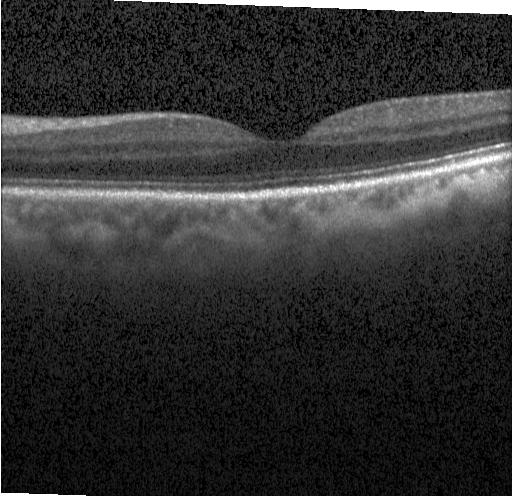
Spectral-domain optical coherence tomography, horizontal scan through the fovea, retinal OCT B-scan
Finding: no evidence of choroidal neovascularization, diabetic macular edema, or drusen.